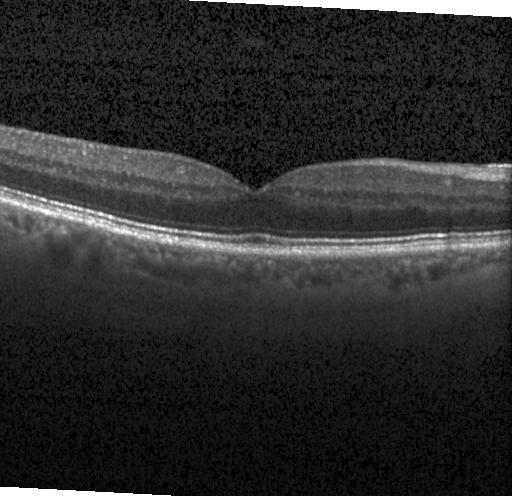
Horizontal scan through the fovea. Acquired on a Heidelberg Spectralis. OCT line scan. Macular OCT: neither choroidal neovascularization, diabetic macular edema, nor drusen.